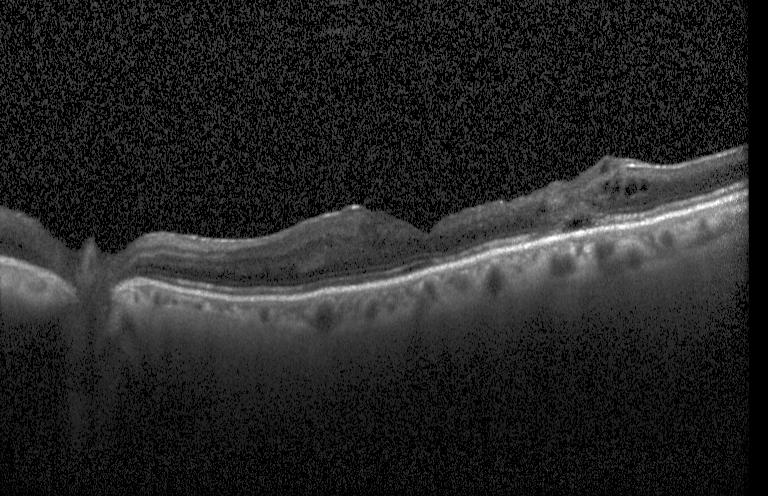
Finding: DME.